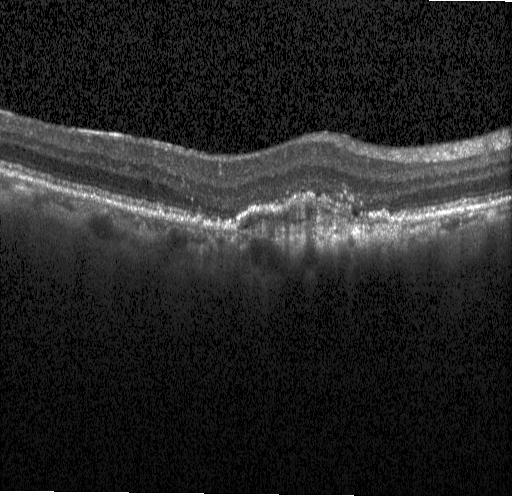

Instrument: Heidelberg Spectralis, centered on the fovea, spectral-domain OCT, retinal OCT B-scan. This B-scan demonstrates choroidal neovascularization (CNV).